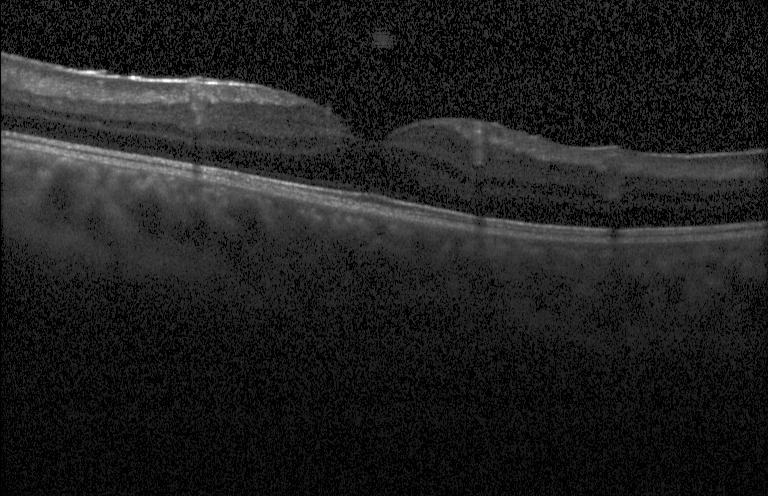
OCT finding: no CNV, DME, or drusen.